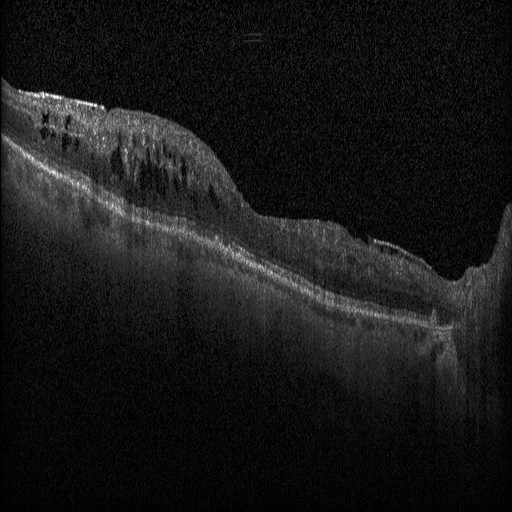

OCT scan showing diabetic macular edema (DME).